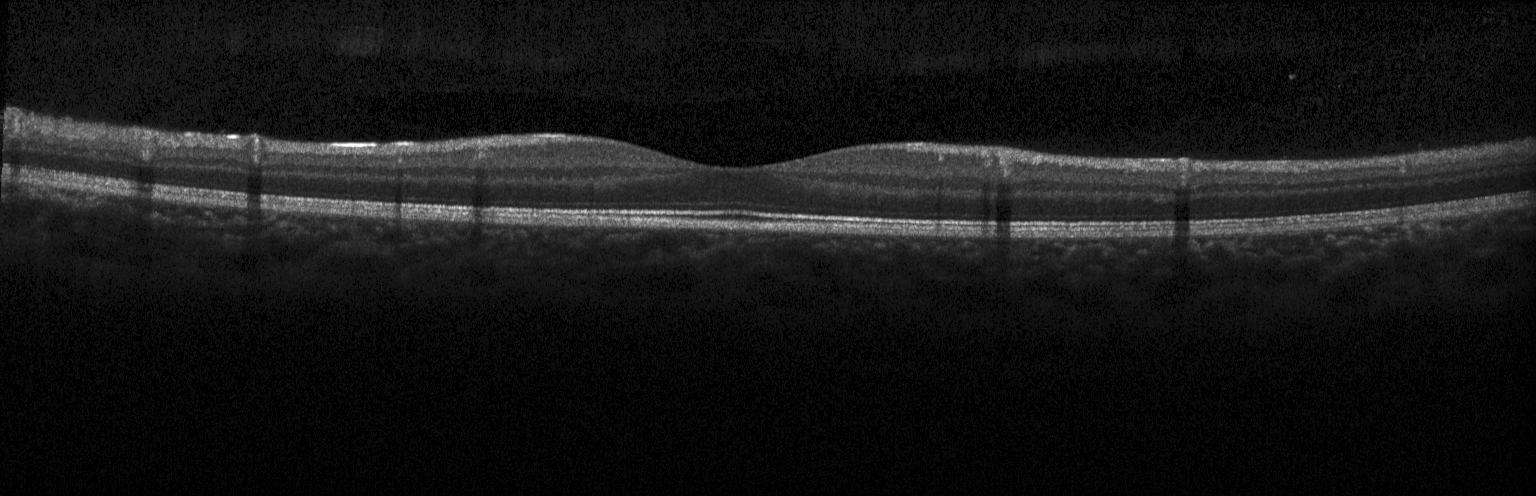 Retinal OCT cross-section showing no evidence of CNV, DME, or drusen.